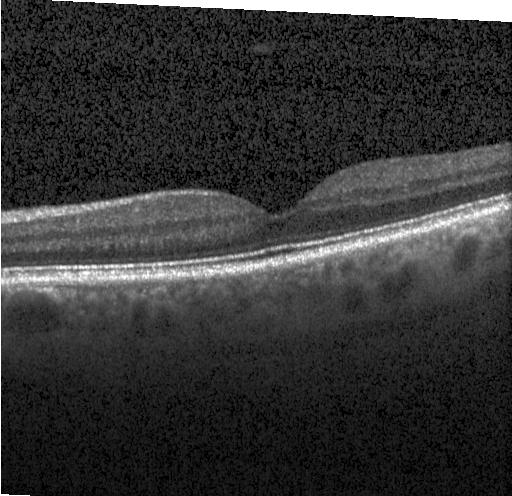 OCT line scan — Impression: neither CNV, DME, nor drusen.